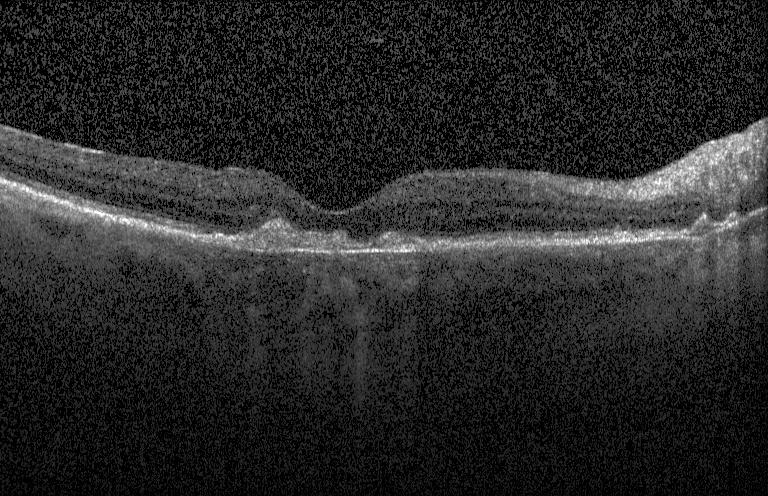 Impression: a choroidal neovascular membrane.